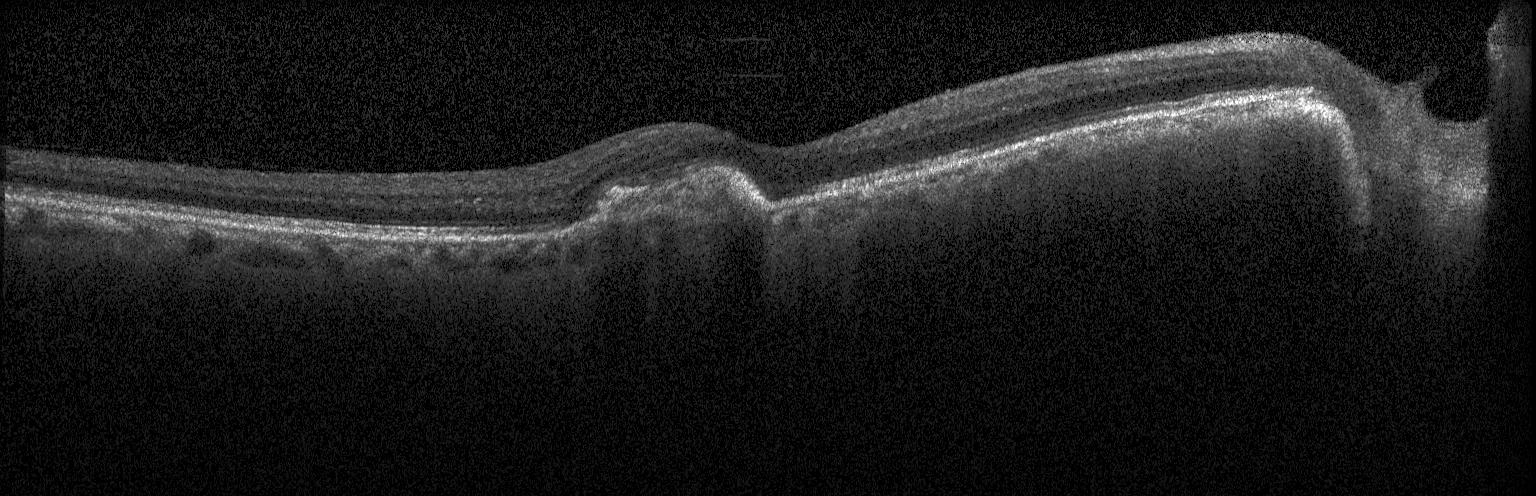

Optical coherence tomography B-scan. Spectral-domain optical coherence tomography. Heidelberg Spectralis. Centered on the fovea. This B-scan demonstrates choroidal neovascularization (CNV).